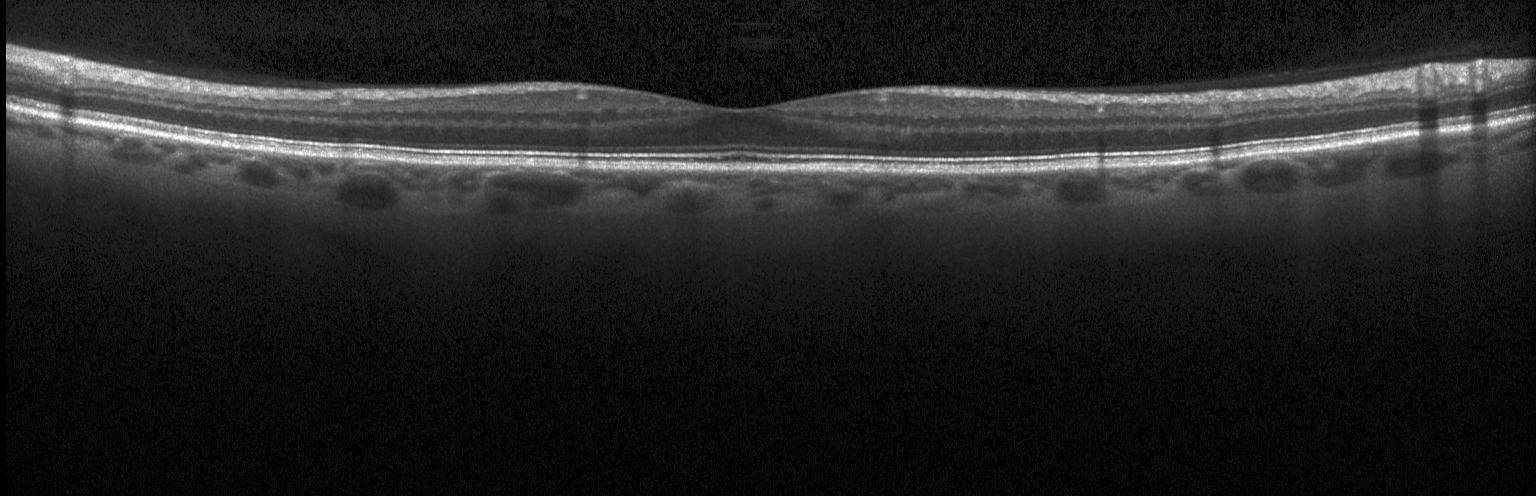
OCT line scan, Heidelberg Spectralis — Finding: no CNV, DME, or drusen.